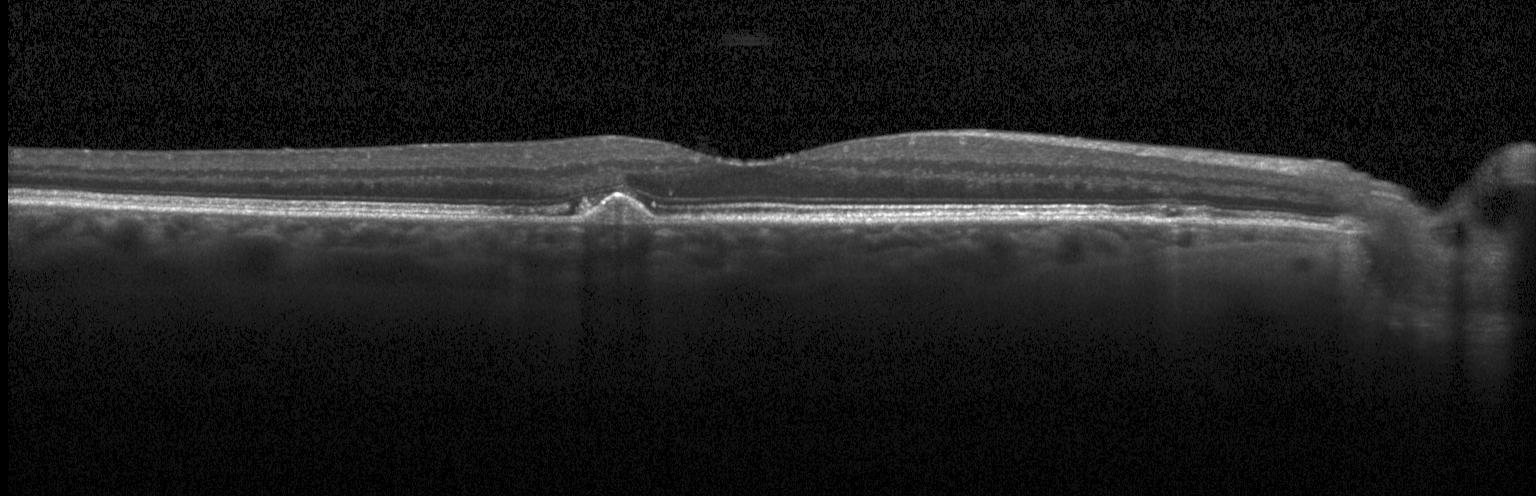 SD-OCT. Optical coherence tomography scan. Acquired on a Heidelberg Spectralis.
This B-scan demonstrates a choroidal neovascular membrane.